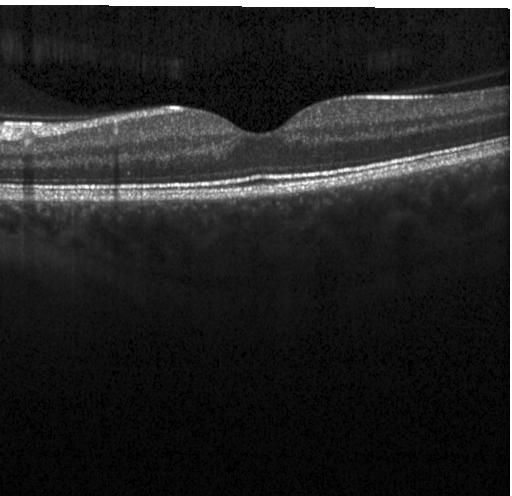
Heidelberg Spectralis OCT system. OCT B-scan
Dx: no evidence of choroidal neovascularization, diabetic macular edema, or drusen.